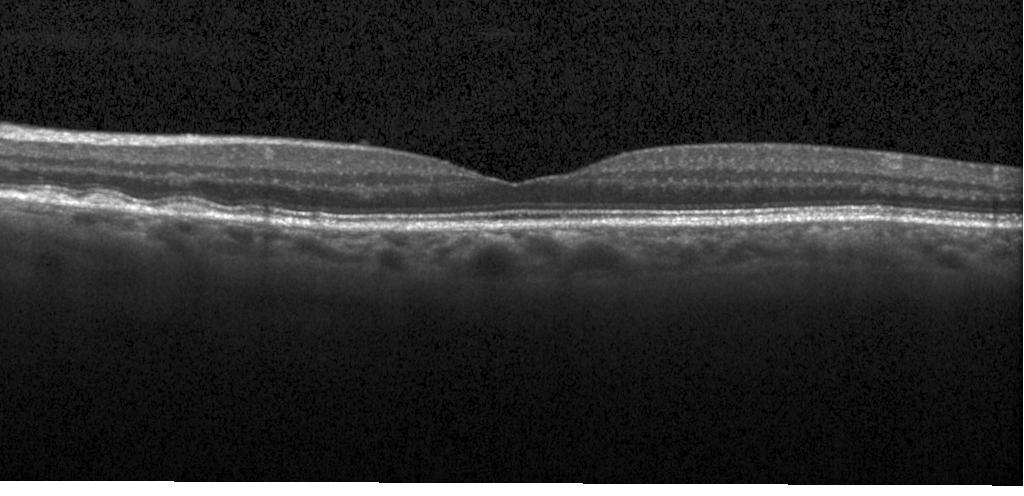

Diagnosis: sub-RPE drusenoid deposits.